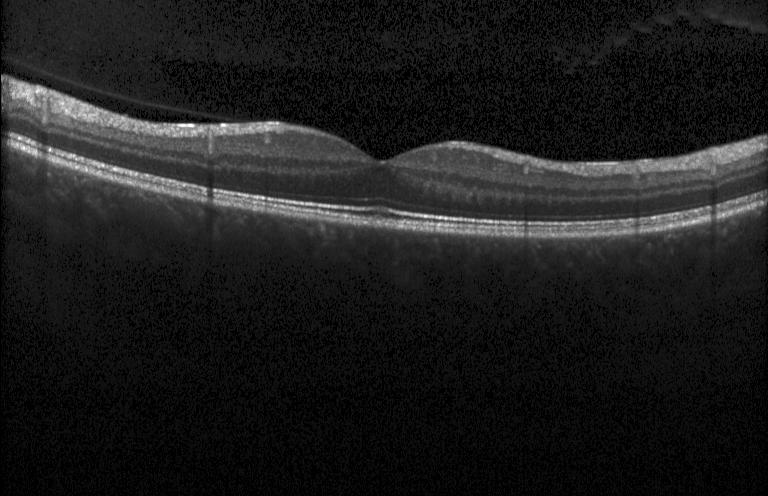 Diagnosis: neither choroidal neovascularization, diabetic macular edema, nor drusen.